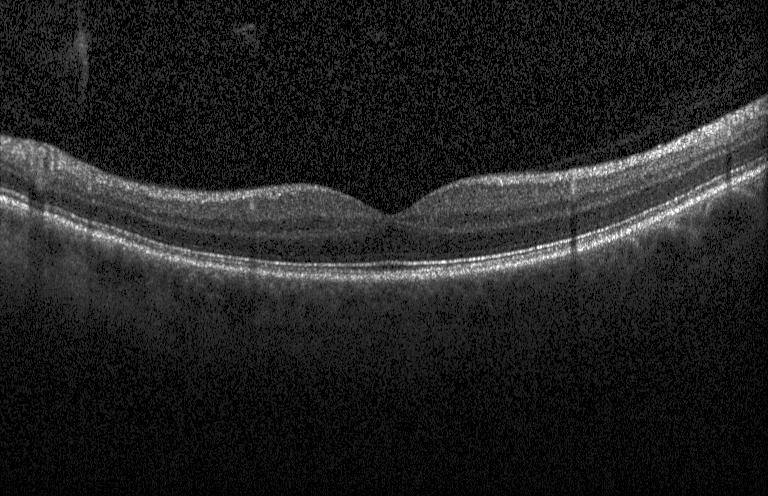
OCT scan showing neither choroidal neovascularization, diabetic macular edema, nor drusen.